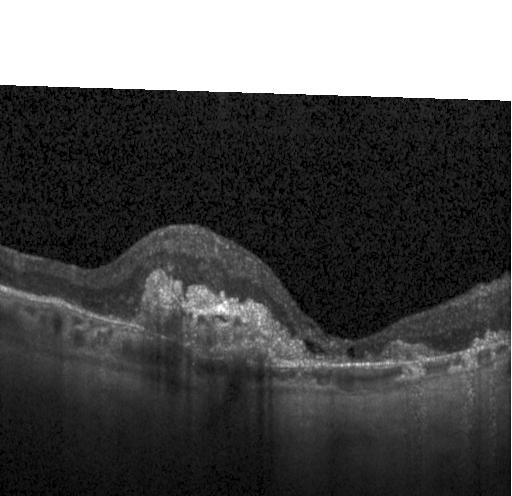 OCT B-scan · through the macula · Heidelberg Spectralis OCT system.
Finding: a choroidal neovascular membrane.